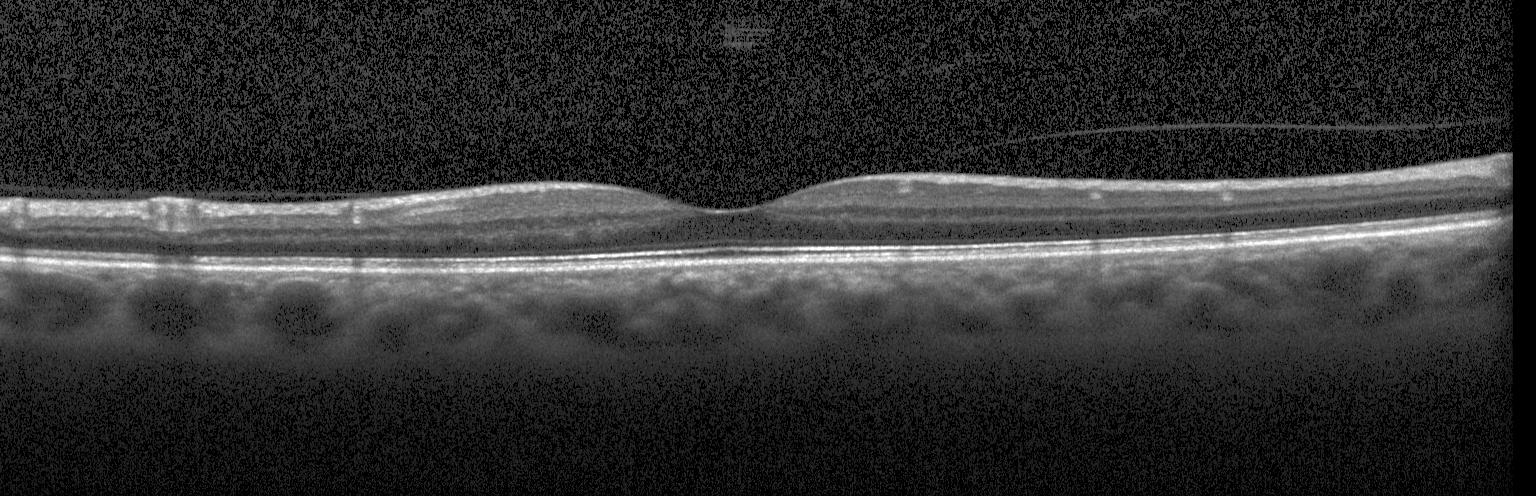

OCT B-scan. Through the macula. Acquired on a Heidelberg Spectralis
Assessment: no evidence of CNV, DME, or drusen.